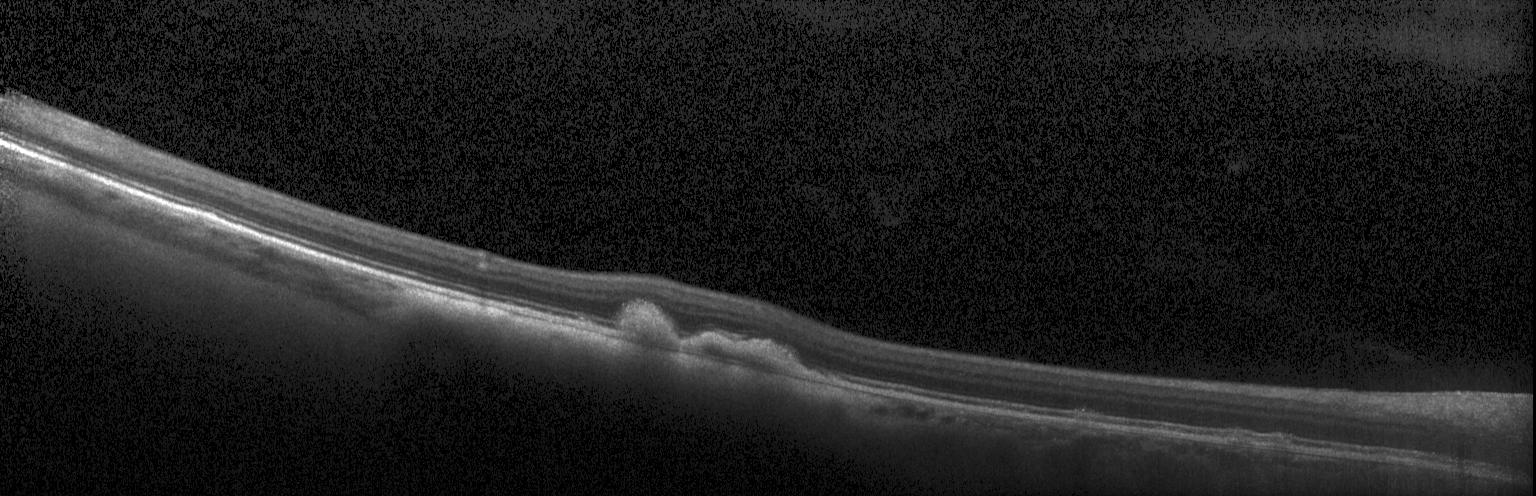
Spectral-domain OCT B-scan: choroidal neovascularization (CNV).